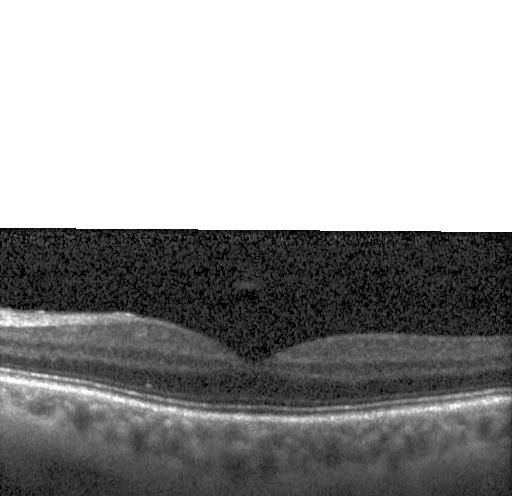

Retinal OCT B-scan · Heidelberg Spectralis OCT system — Diagnosis: no choroidal neovascularization, no diabetic macular edema, and no drusen.